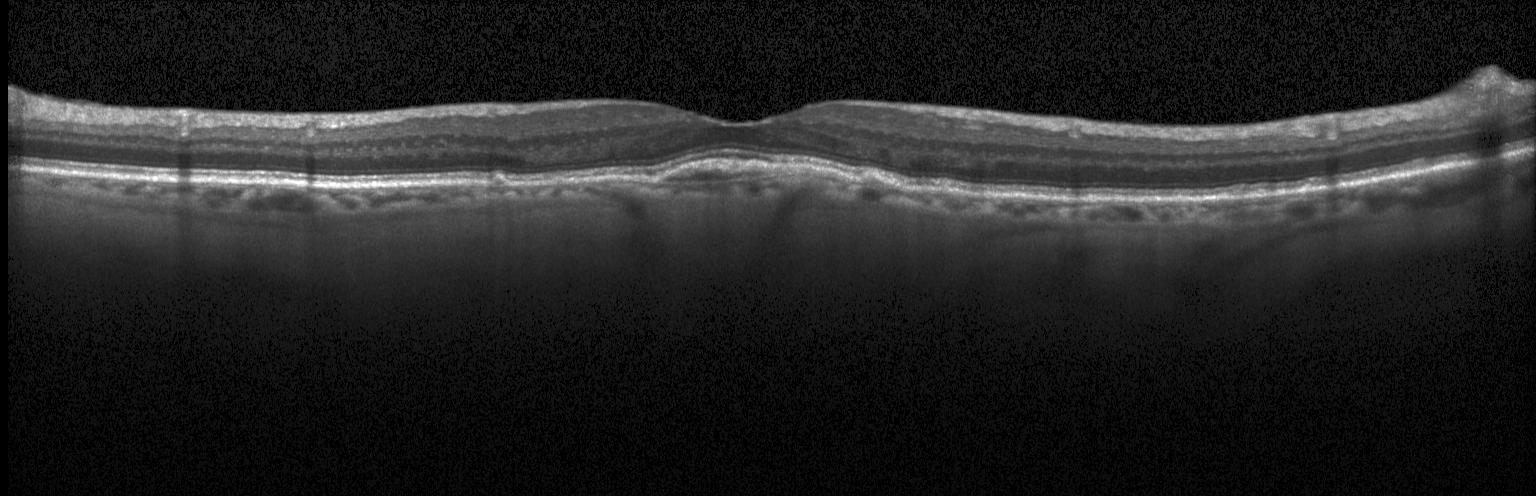

OCT scan showing a choroidal neovascular membrane.